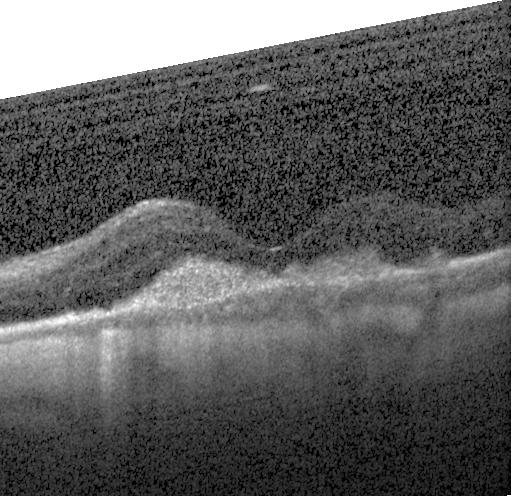 Optical coherence tomography B-scan; fovea-centered; SD-OCT. Impression: choroidal neovascularization.